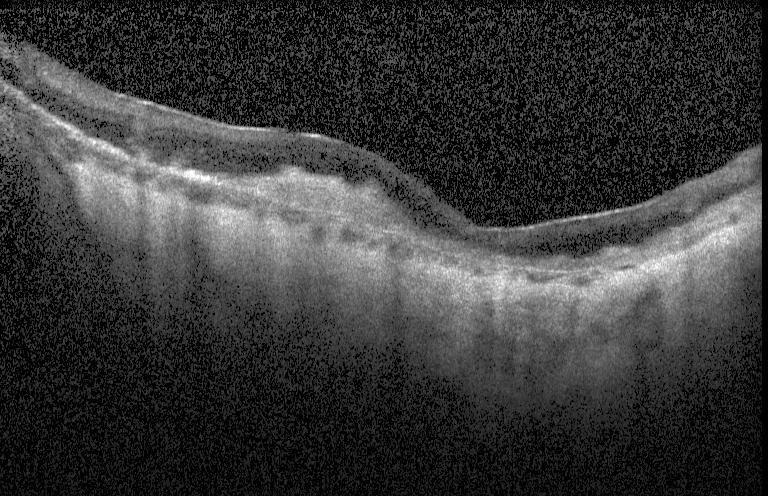

Heidelberg Spectralis OCT system; retinal OCT B-scan — The scan shows a choroidal neovascular membrane.